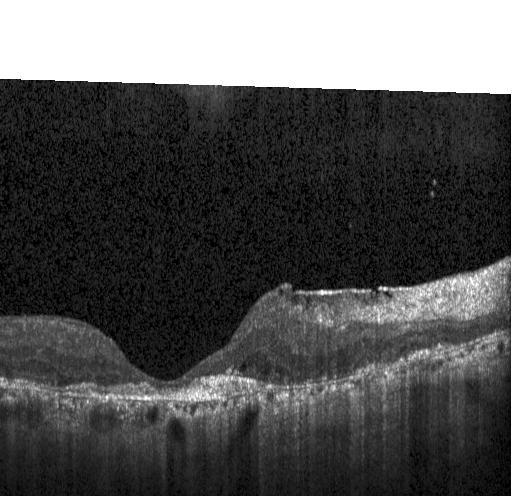

Retinal OCT B-scan.
Assessment: CNV.